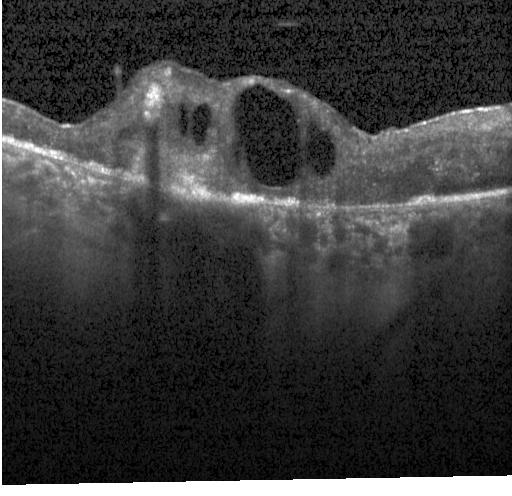

Spectral-domain OCT B-scan: a choroidal neovascular membrane.